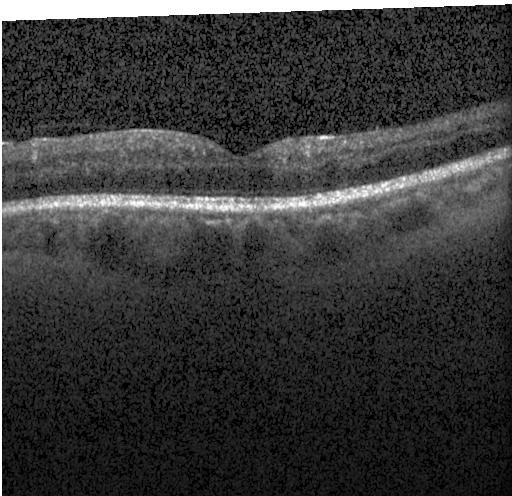 Fovea-centered, retinal OCT B-scan
No choroidal neovascularization, diabetic macular edema, or drusen.